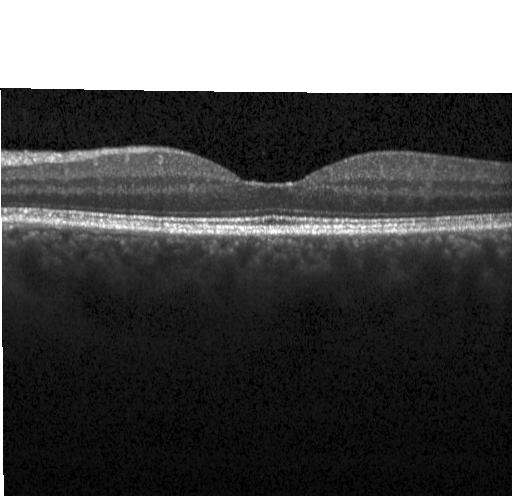

OCT finding: no choroidal neovascularization, no diabetic macular edema, and no drusen.